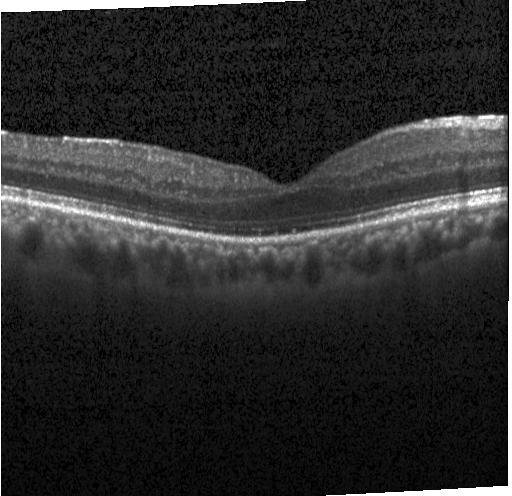
No choroidal neovascularization, no diabetic macular edema, and no drusen.